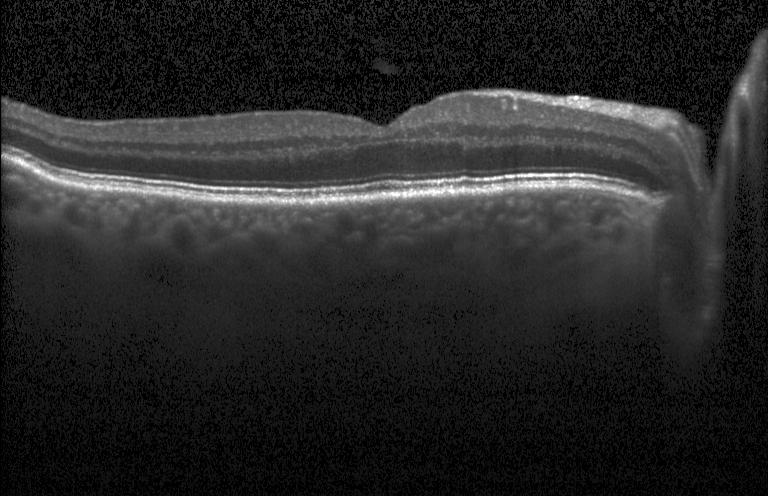

Optical coherence tomography scan, through the macula — OCT finding: neither CNV, DME, nor drusen.